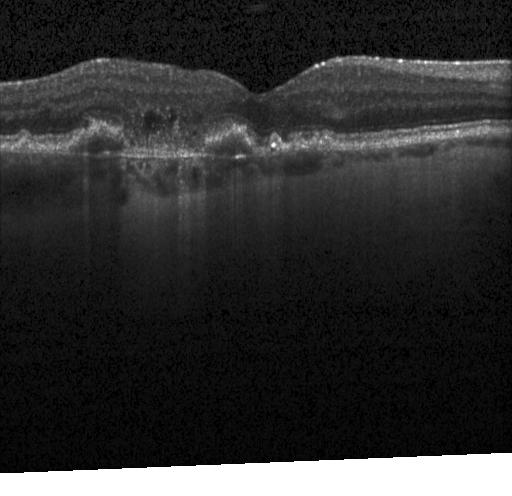
Impression: a choroidal neovascular membrane.